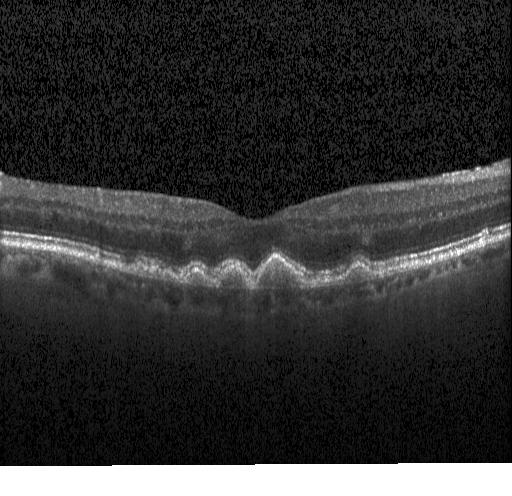
OCT line scan — Finding: drusen.